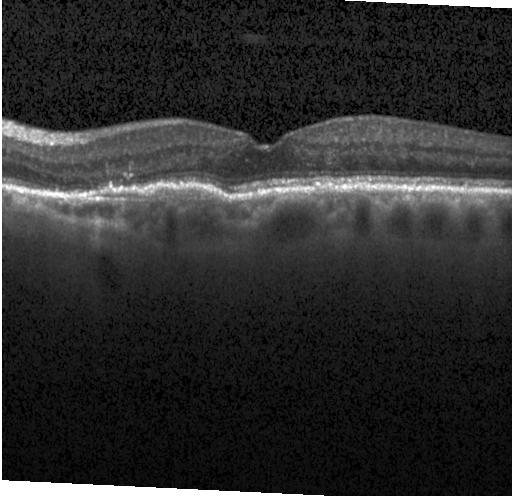 Optical coherence tomography B-scan; spectral-domain optical coherence tomography.
Dx: choroidal neovascularization (CNV).